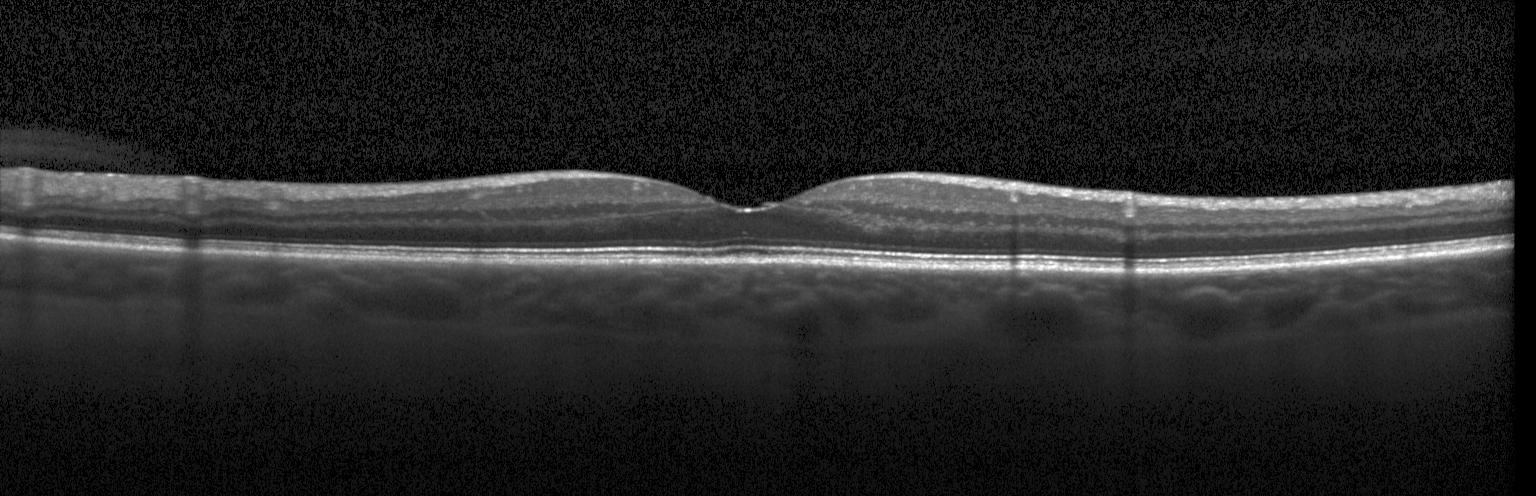
Spectral-domain OCT, macular scan, optical coherence tomography B-scan — OCT finding: no choroidal neovascularization, no diabetic macular edema, and no drusen.